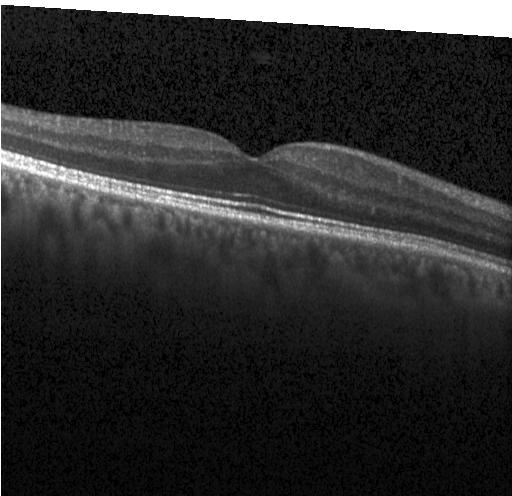
Optical coherence tomography B-scan
Assessment: no evidence of choroidal neovascularization, diabetic macular edema, or drusen.